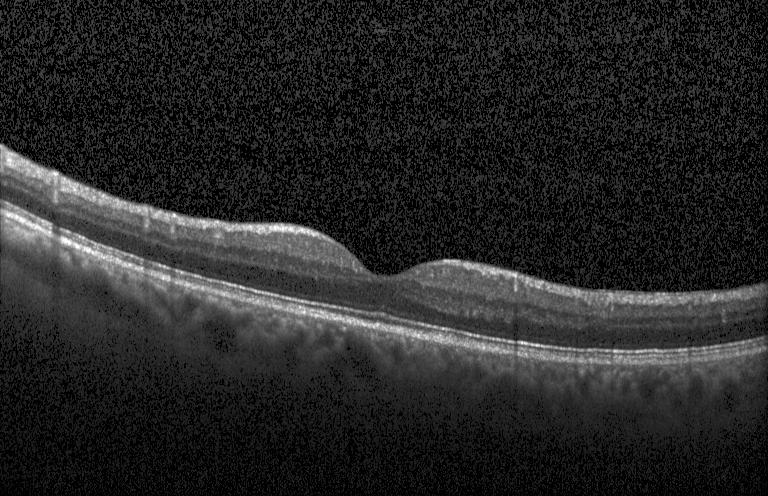 Retinal OCT B-scan — Macular OCT: no choroidal neovascularization, no diabetic macular edema, and no drusen.